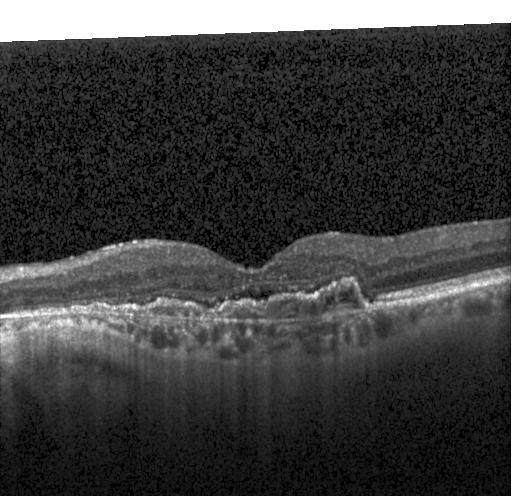 OCT line scan; Heidelberg Spectralis OCT system
OCT finding: choroidal neovascularization (CNV).